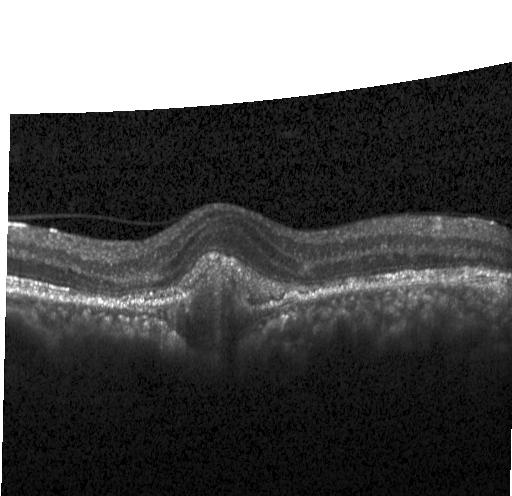

Optical coherence tomography scan — Diagnosis: choroidal neovascularization (CNV).